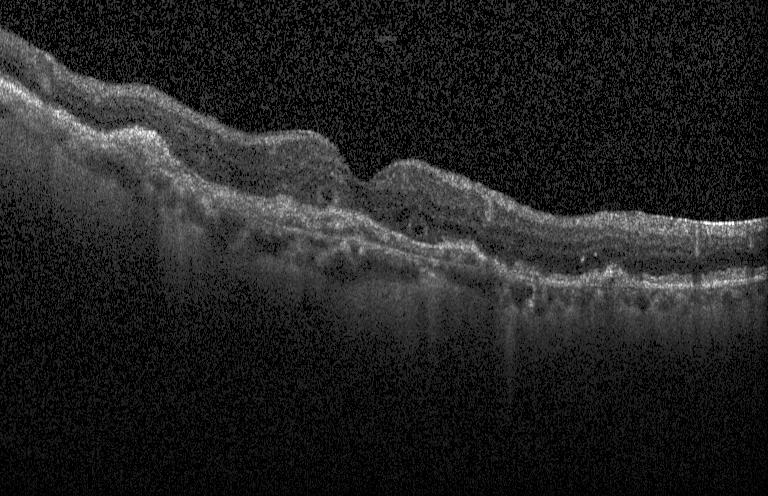
OCT scan showing a choroidal neovascular membrane.